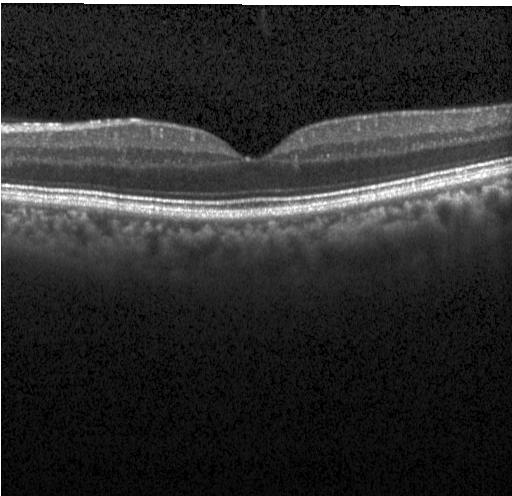
Heidelberg Spectralis OCT system, spectral-domain optical coherence tomography, fovea-centered, retinal OCT cross-section.
The scan shows no choroidal neovascularization, diabetic macular edema, or drusen.